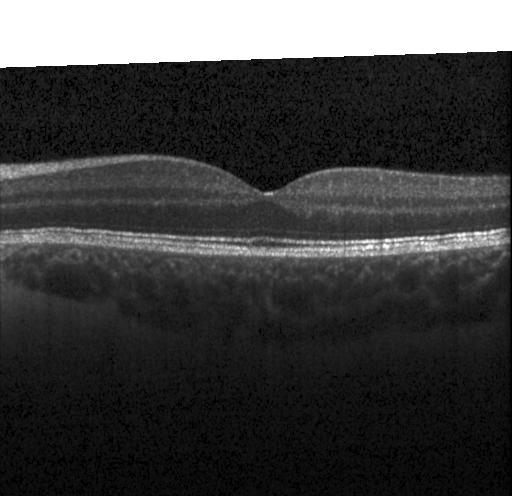 OCT finding: no choroidal neovascularization, diabetic macular edema, or drusen.